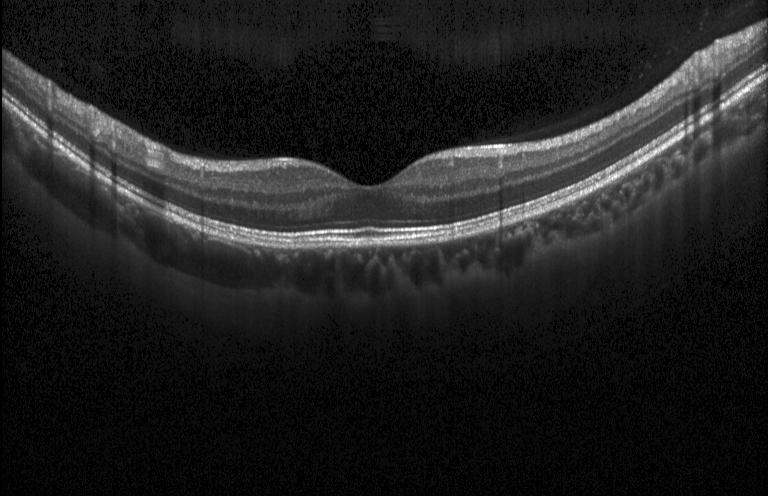

OCT scan showing no choroidal neovascularization, diabetic macular edema, or drusen.